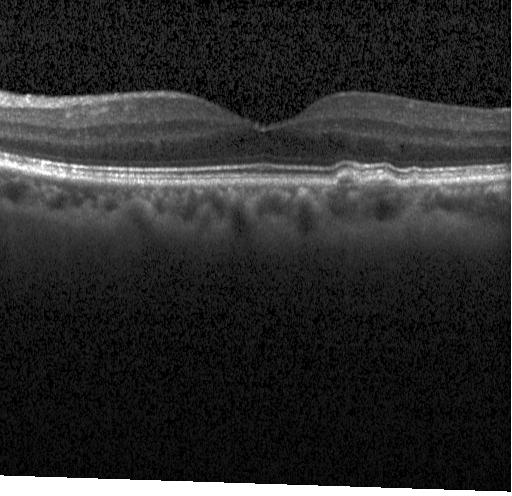

Spectral-domain OCT. Optical coherence tomography scan. Fovea-centered. Heidelberg Spectralis. Diagnosis: multiple drusen.